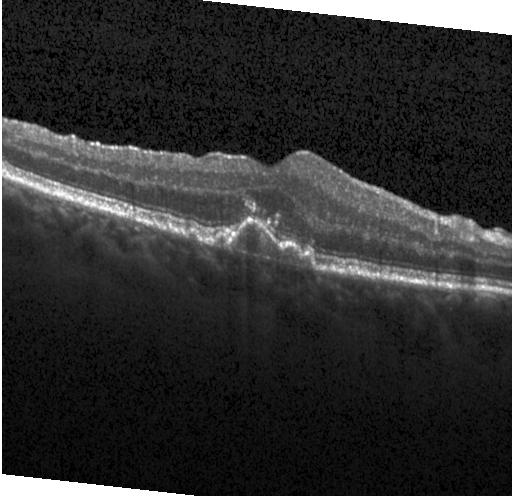 Finding: sub-RPE drusenoid deposits.